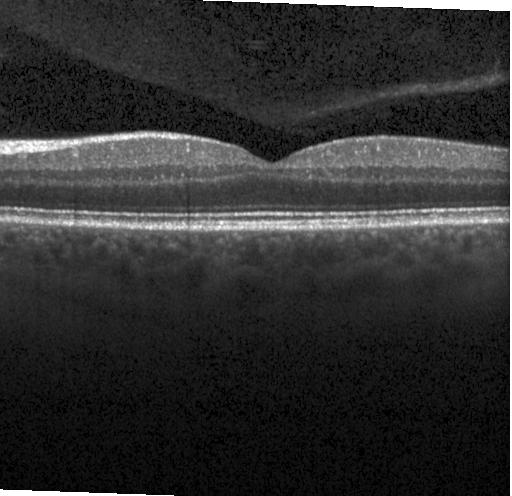 OCT B-scan, macular scan. Finding: no choroidal neovascularization, no diabetic macular edema, and no drusen.